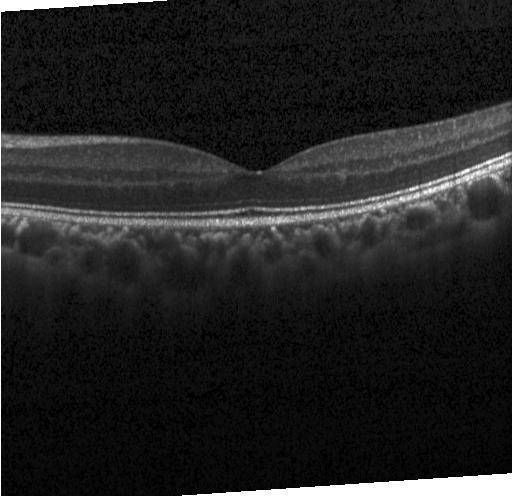
Optical coherence tomography B-scan — The scan shows neither choroidal neovascularization, diabetic macular edema, nor drusen.